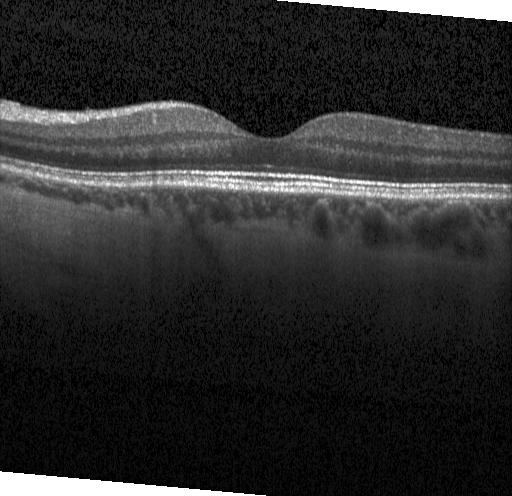

OCT B-scan showing no choroidal neovascularization, no diabetic macular edema, and no drusen.